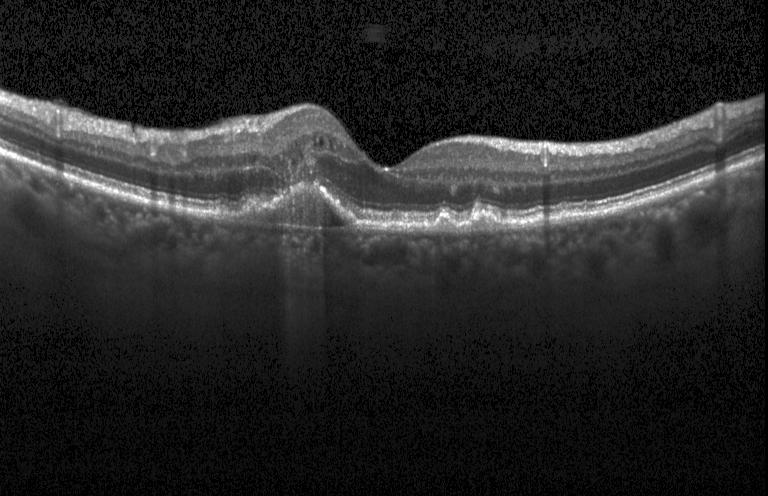
Diagnosis: choroidal neovascularization (CNV).